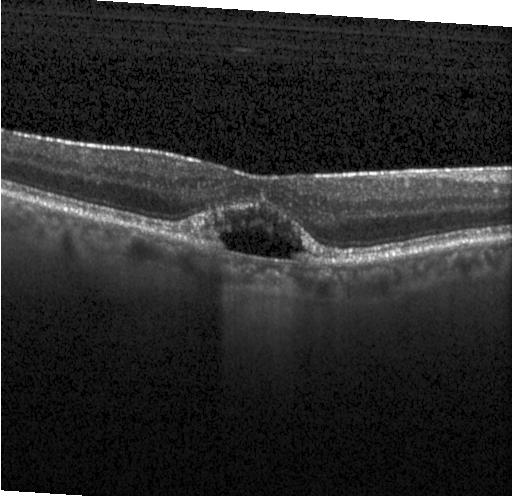 Retinal OCT B-scan, acquired on a Heidelberg Spectralis, macular scan, spectral-domain OCT
Impression: choroidal neovascularization (CNV).